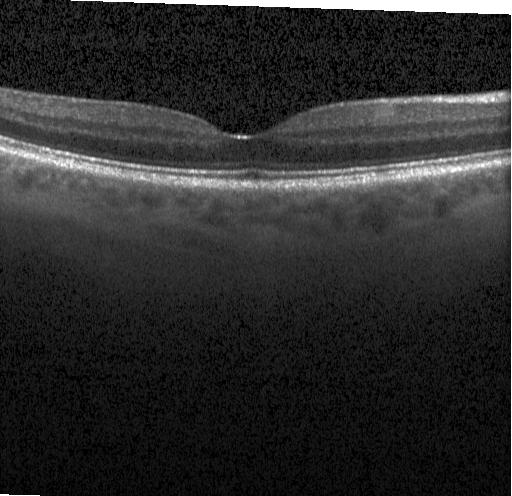

OCT line scan; macular scan. Macular OCT: neither choroidal neovascularization, diabetic macular edema, nor drusen.